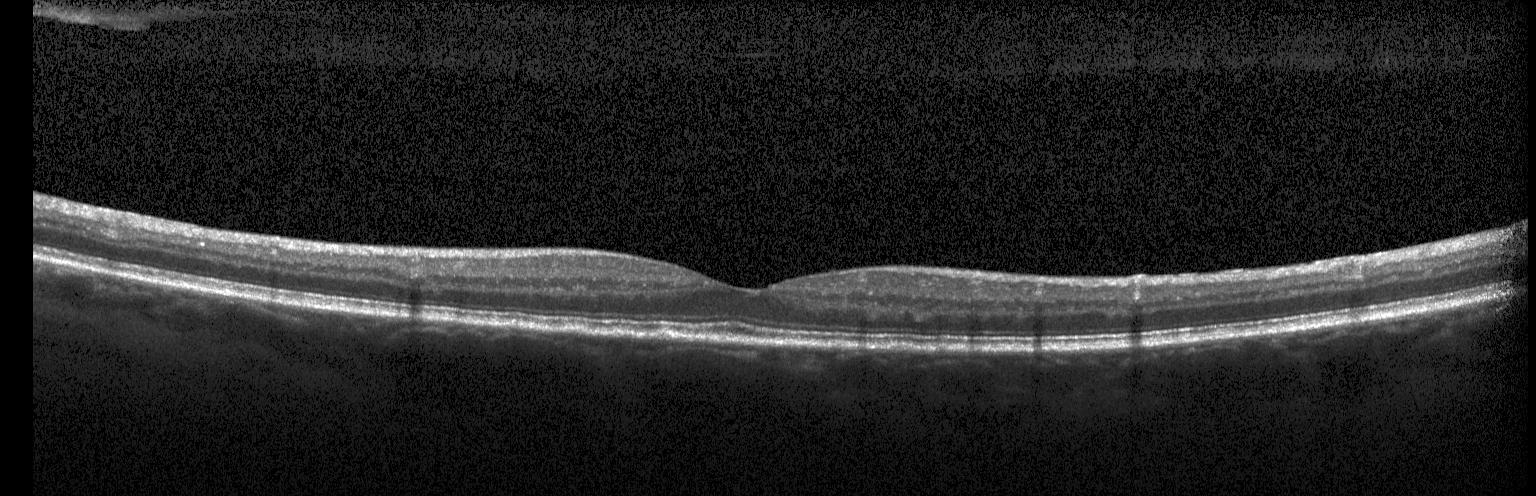
Retinal OCT cross-section, Heidelberg Spectralis. OCT finding: no choroidal neovascularization, diabetic macular edema, or drusen.